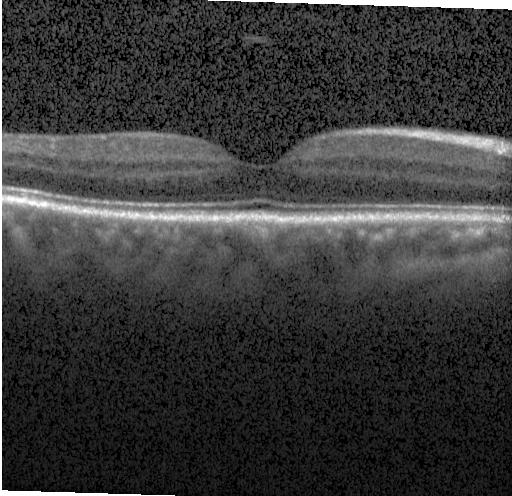 SD-OCT. Fovea-centered. Heidelberg Spectralis. Optical coherence tomography scan
Assessment: neither choroidal neovascularization, diabetic macular edema, nor drusen.